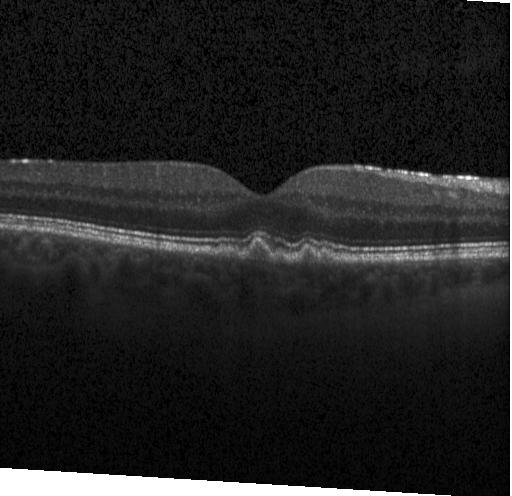 Macular OCT: sub-RPE drusenoid deposits.